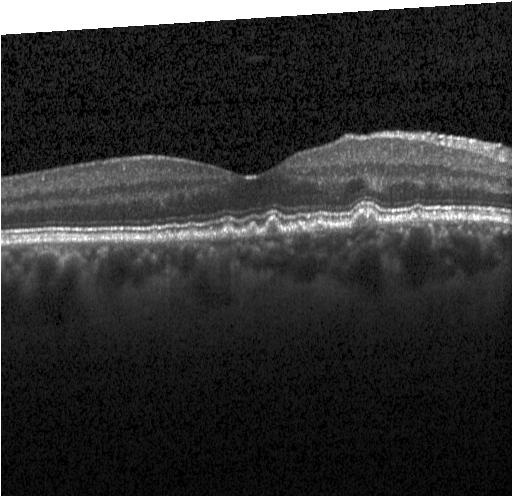
Retinal OCT B-scan · Heidelberg Spectralis OCT system · centered on the fovea · spectral-domain optical coherence tomography
Assessment: sub-RPE drusenoid deposits.